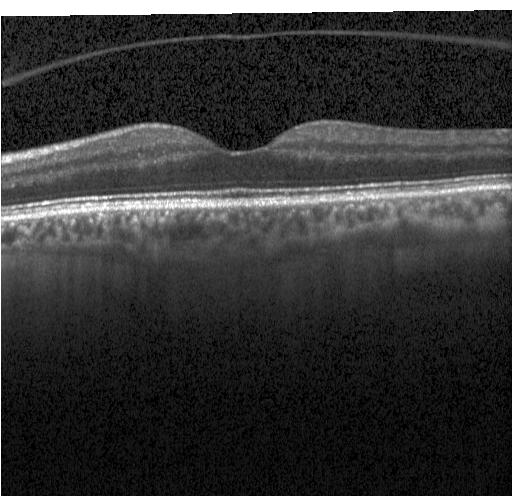

OCT B-scan.
Macular OCT: neither choroidal neovascularization, diabetic macular edema, nor drusen.